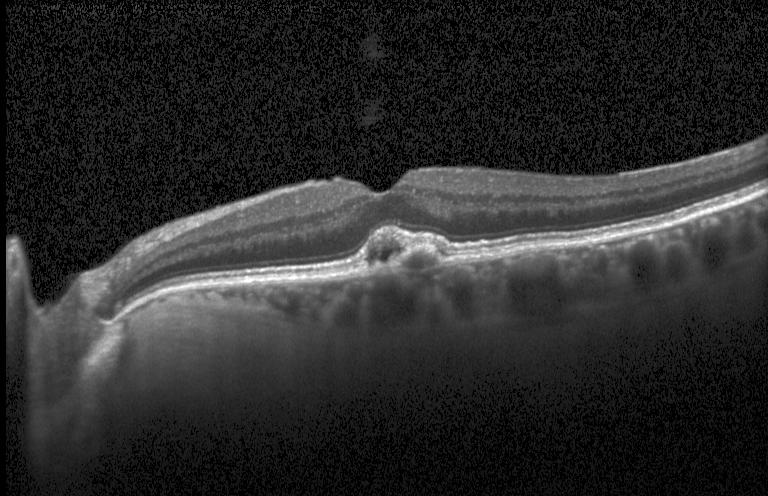

Optical coherence tomography B-scan. Through the macula.
Diagnosis: a choroidal neovascular membrane.